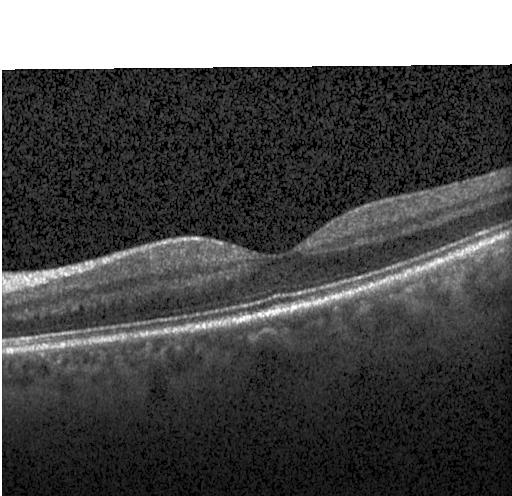
The scan shows no evidence of choroidal neovascularization, diabetic macular edema, or drusen.